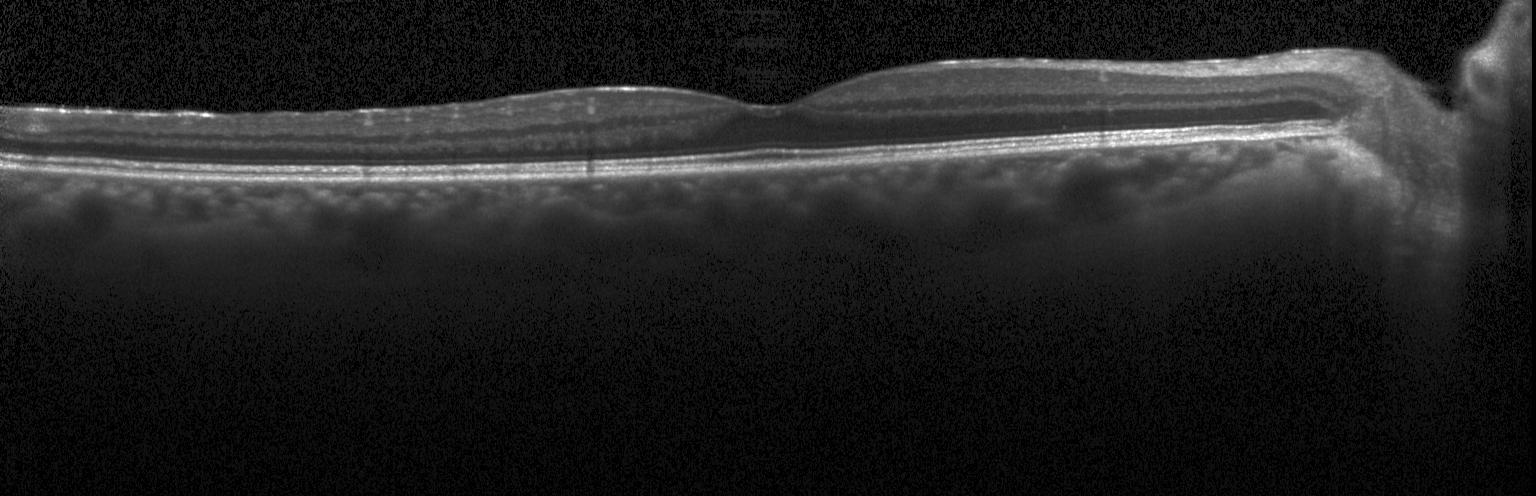
OCT line scan · macular scan · SD-OCT. Neither CNV, DME, nor drusen.